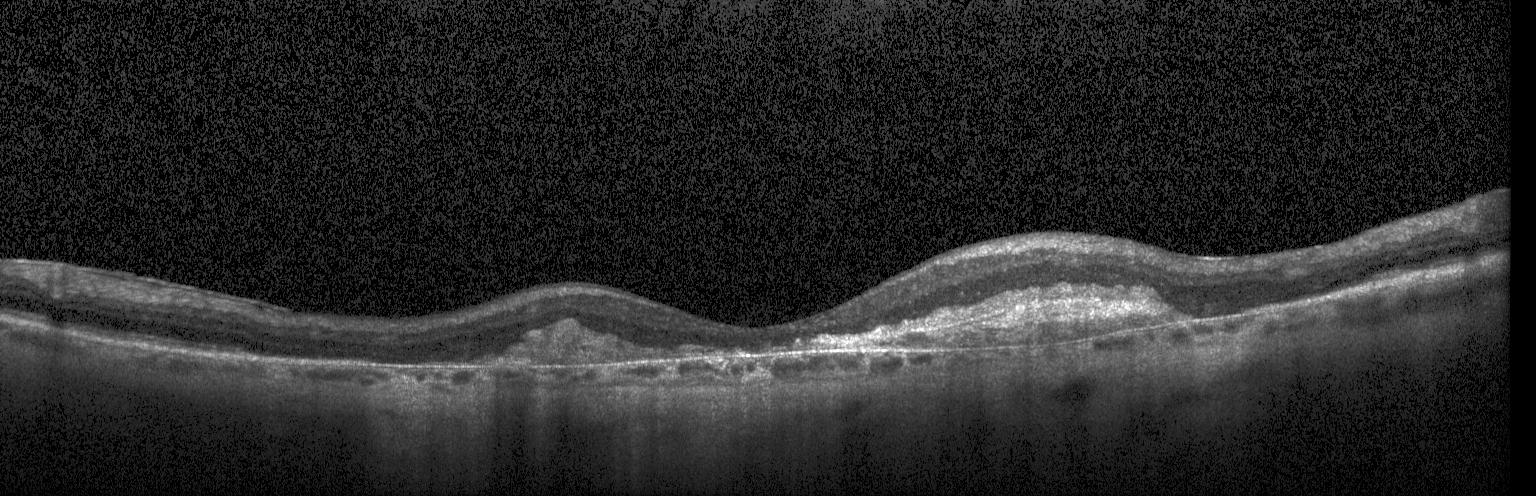

Finding: choroidal neovascularization.